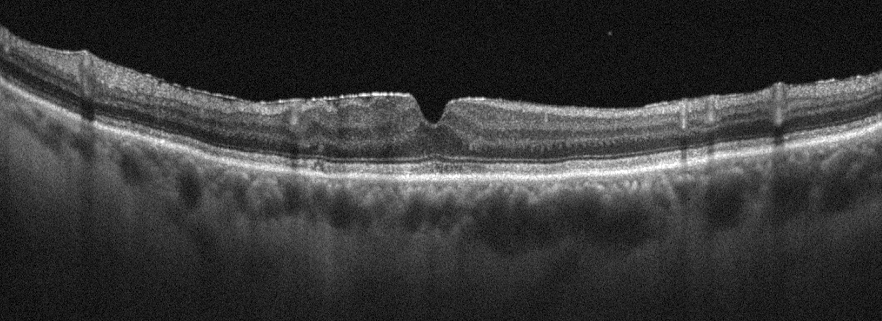

Spectral-domain OCT B-scan: epiretinal membrane (ERM).